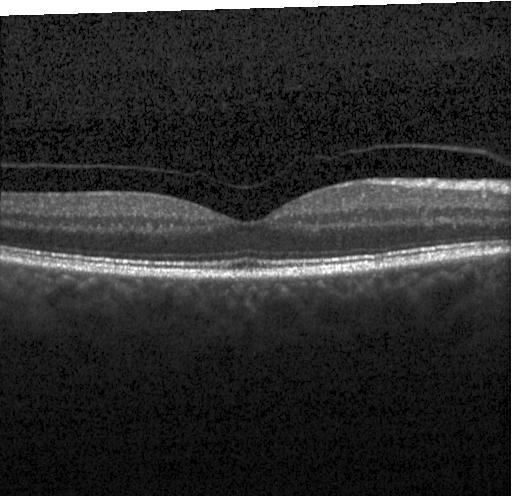

Finding: neither choroidal neovascularization, diabetic macular edema, nor drusen.